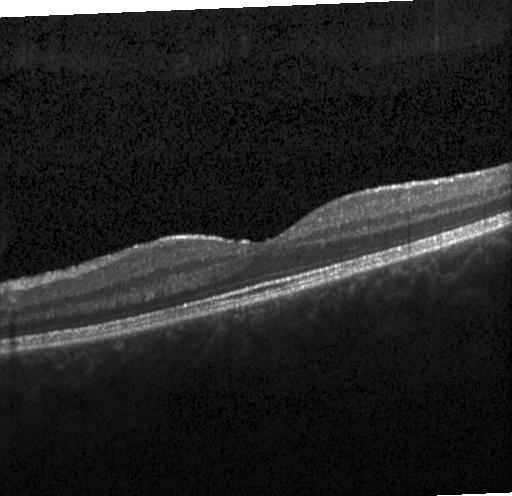 Impression: no choroidal neovascularization, no diabetic macular edema, and no drusen.